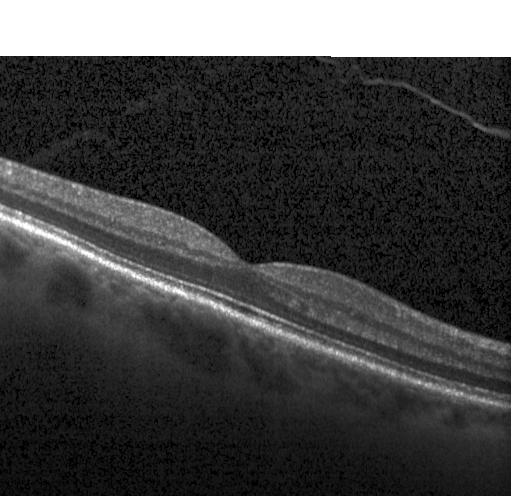 SD-OCT; Heidelberg Spectralis OCT system; fovea-centered; optical coherence tomography scan — This B-scan demonstrates no choroidal neovascularization, no diabetic macular edema, and no drusen.